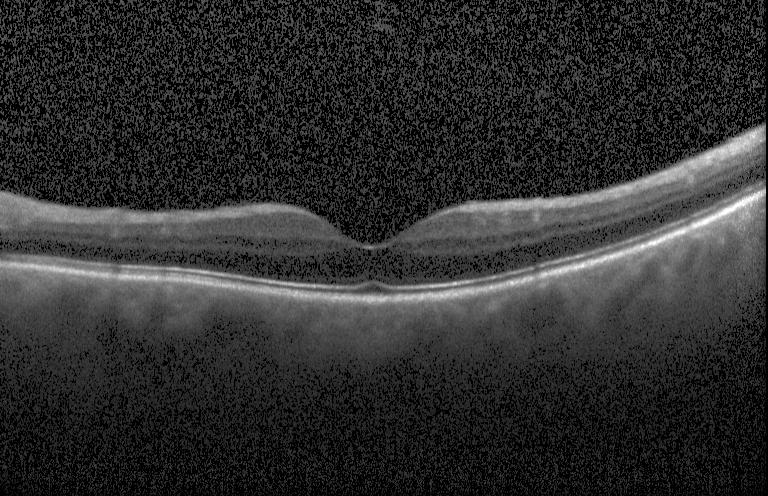

Heidelberg Spectralis. Through the macula. OCT B-scan
Neither choroidal neovascularization, diabetic macular edema, nor drusen.